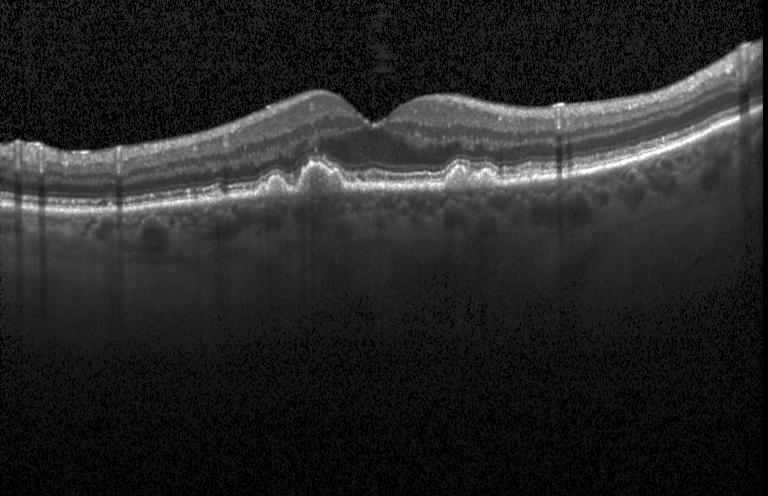

Impression: sub-RPE drusenoid deposits.